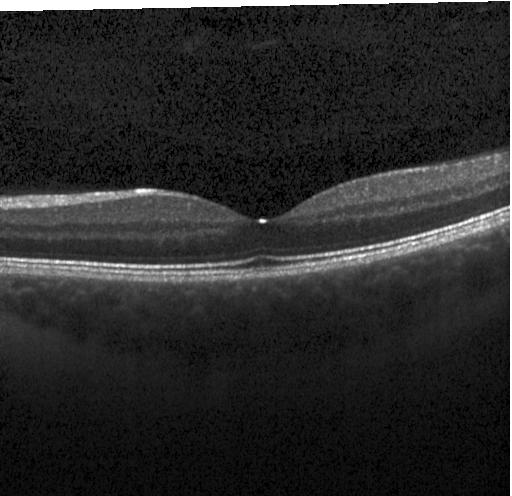 This B-scan demonstrates neither choroidal neovascularization, diabetic macular edema, nor drusen.